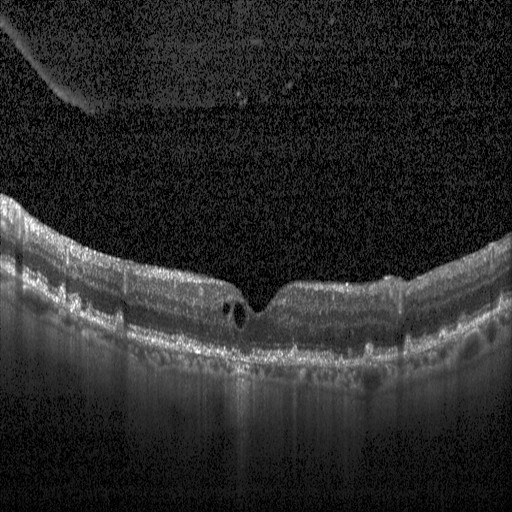

Dx: DME.